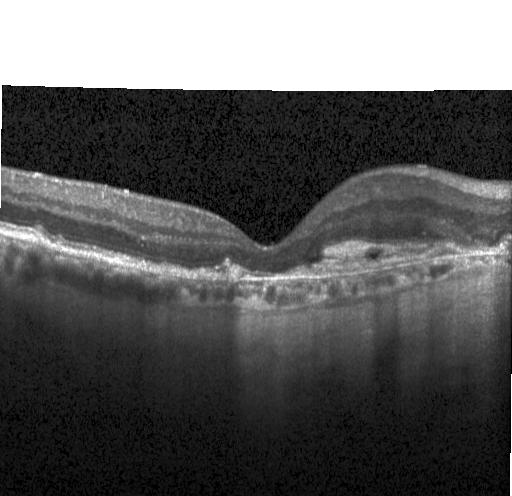
Retinal OCT B-scan.
Diagnosis: a choroidal neovascular membrane.